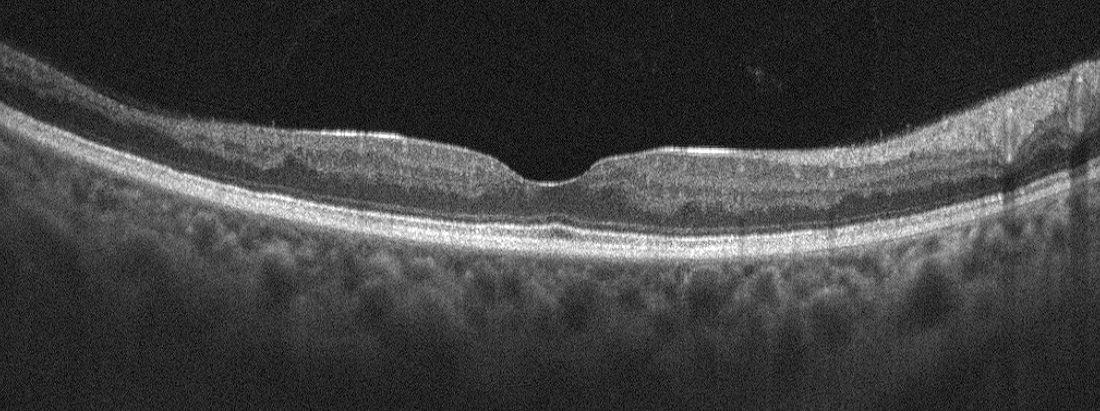

Macular OCT: retinal vein occlusion.